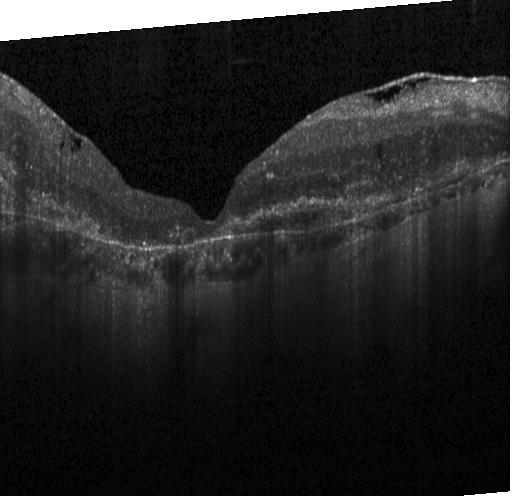 Spectral-domain optical coherence tomography, retinal OCT cross-section, acquired on a Heidelberg Spectralis.
The scan shows CNV.